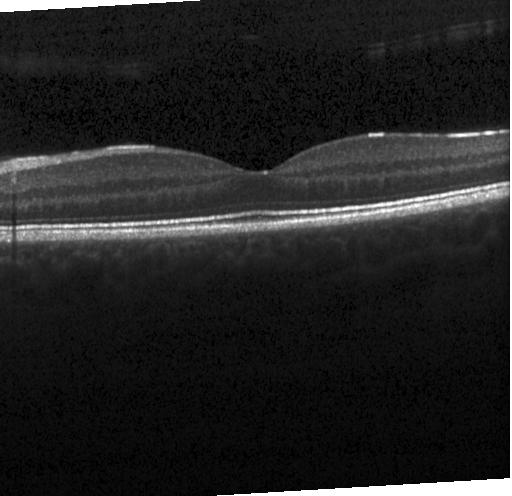 The scan shows neither choroidal neovascularization, diabetic macular edema, nor drusen.